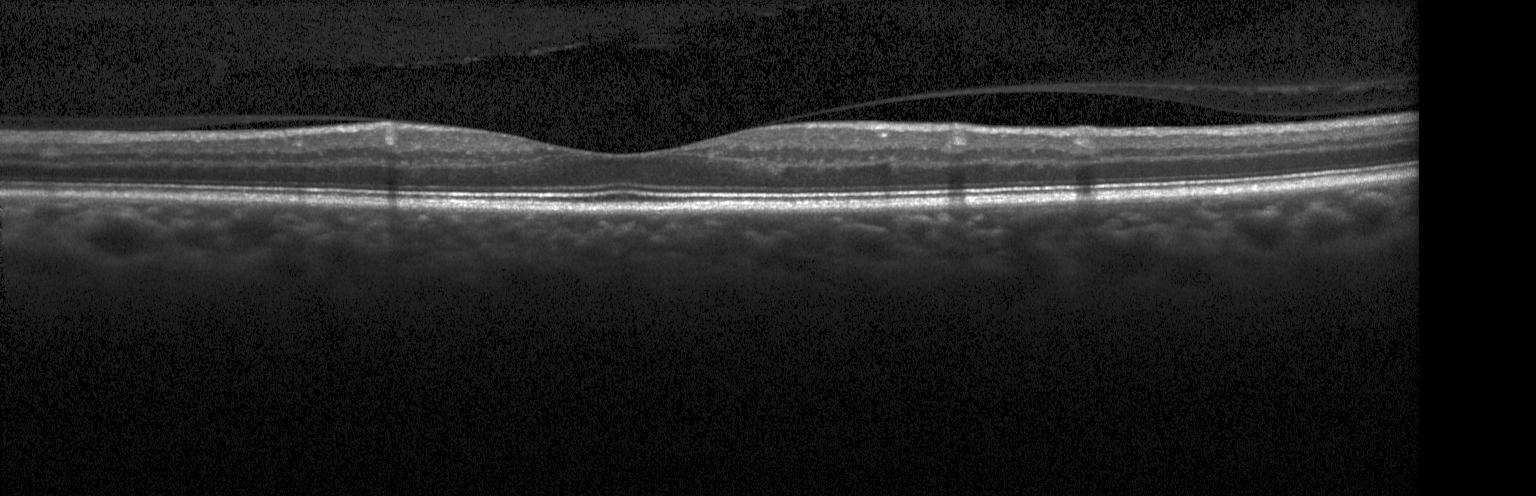

Heidelberg Spectralis, SD-OCT, OCT B-scan, fovea-centered.
This B-scan demonstrates no evidence of choroidal neovascularization, diabetic macular edema, or drusen.